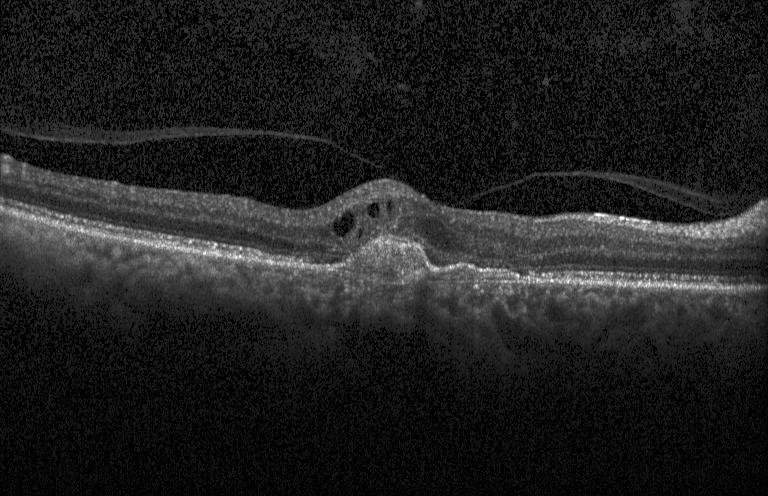

Optical coherence tomography scan — Choroidal neovascularization.